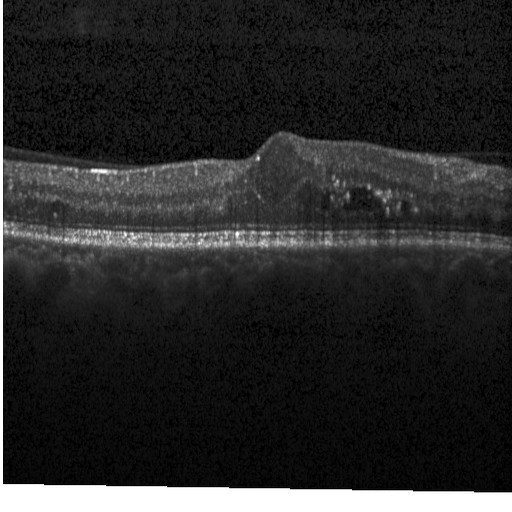 Optical coherence tomography B-scan. Spectral-domain OCT. This B-scan demonstrates DME.